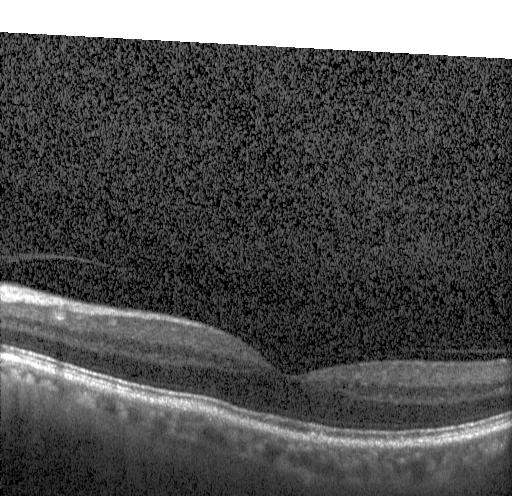
Impression: no choroidal neovascularization, diabetic macular edema, or drusen.